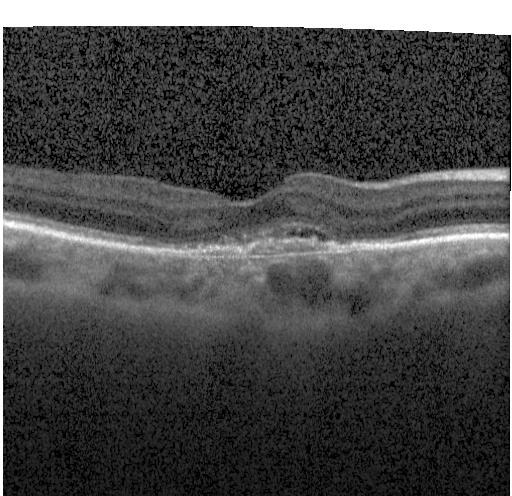

Retinal OCT cross-section. The scan shows a choroidal neovascular membrane.